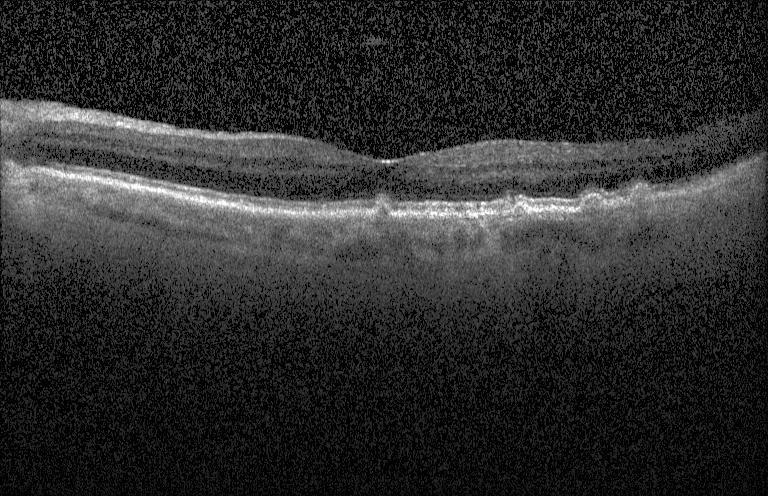
Finding: sub-RPE drusenoid deposits.